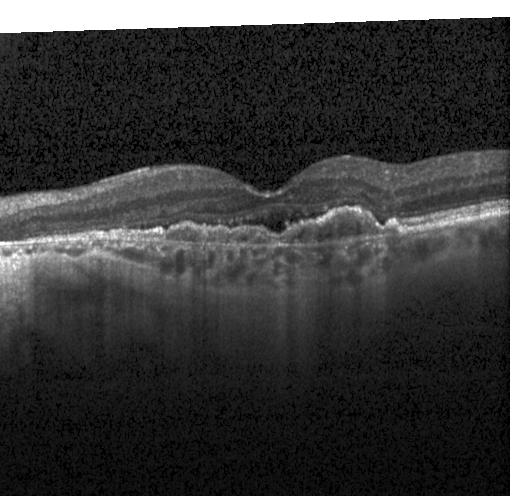

Optical coherence tomography scan.
OCT finding: choroidal neovascularization.